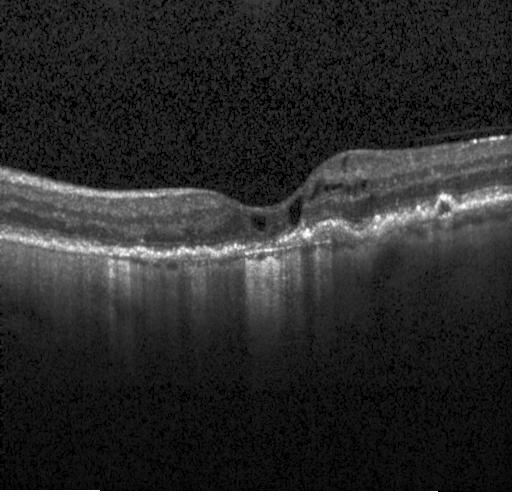
OCT line scan — Impression: CNV.